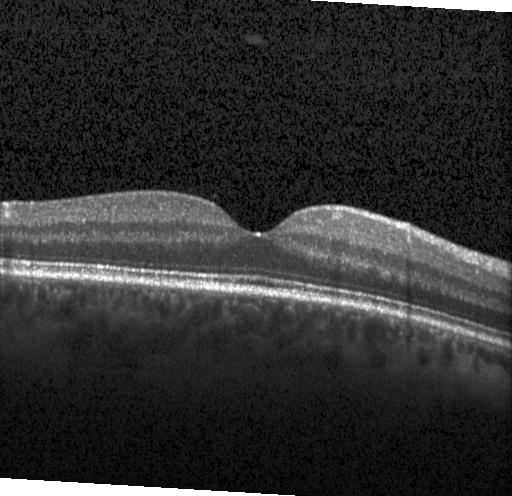 OCT B-scan. Assessment: no evidence of choroidal neovascularization, diabetic macular edema, or drusen.